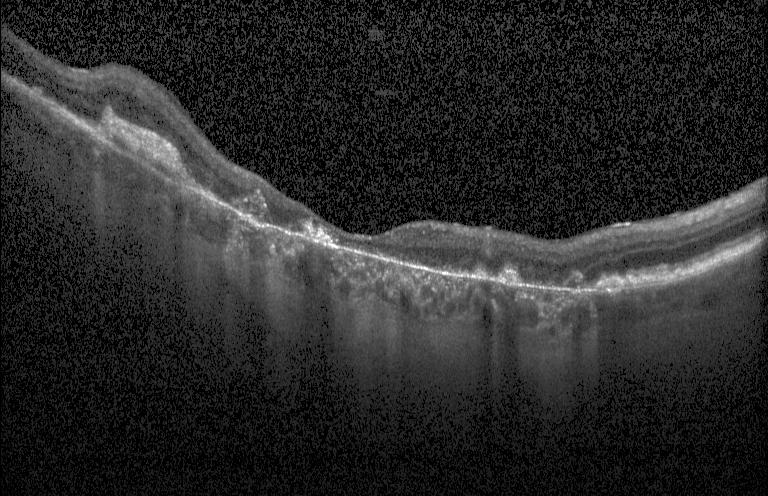
Macular OCT demonstrating CNV.